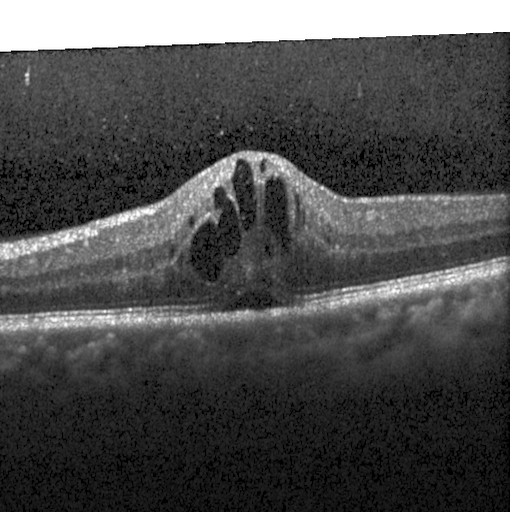

Macular OCT demonstrating DME.